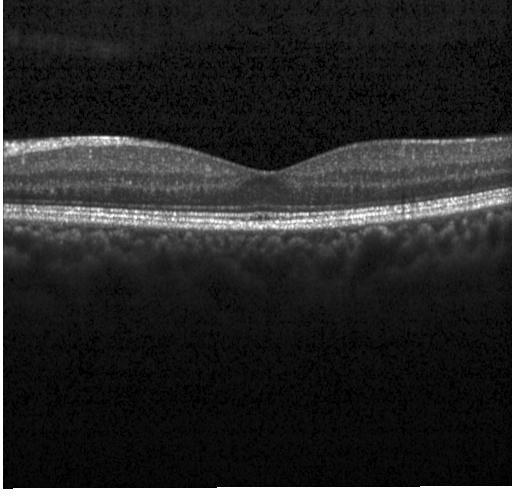

Heidelberg Spectralis OCT system · OCT B-scan · through the macula · spectral-domain optical coherence tomography.
Impression: no choroidal neovascularization, diabetic macular edema, or drusen.